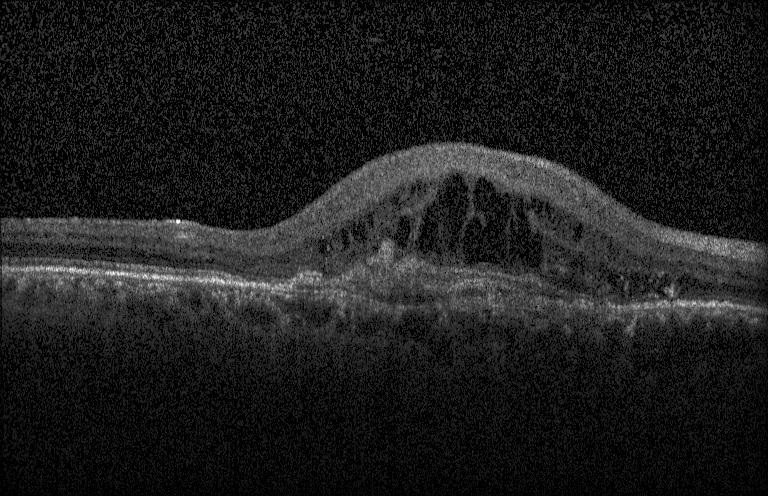

Fovea-centered, optical coherence tomography scan. Diagnosis: choroidal neovascularization (CNV).